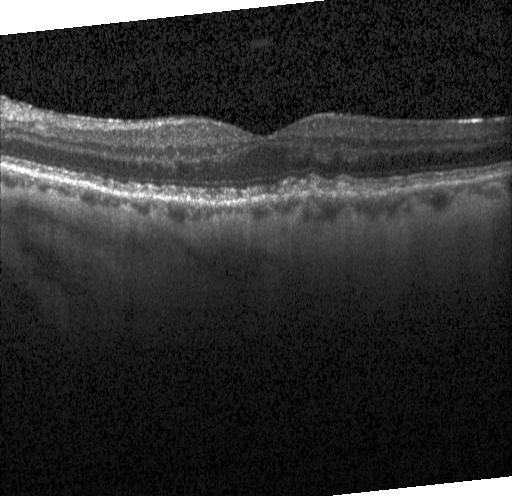
OCT B-scan.
Finding: sub-RPE drusenoid deposits.